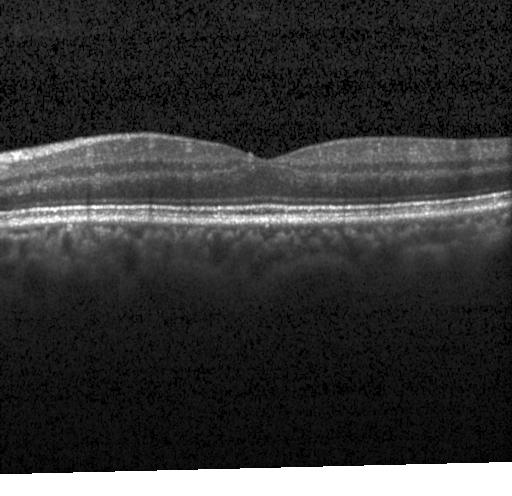 Optical coherence tomography B-scan.
Finding: no evidence of choroidal neovascularization, diabetic macular edema, or drusen.